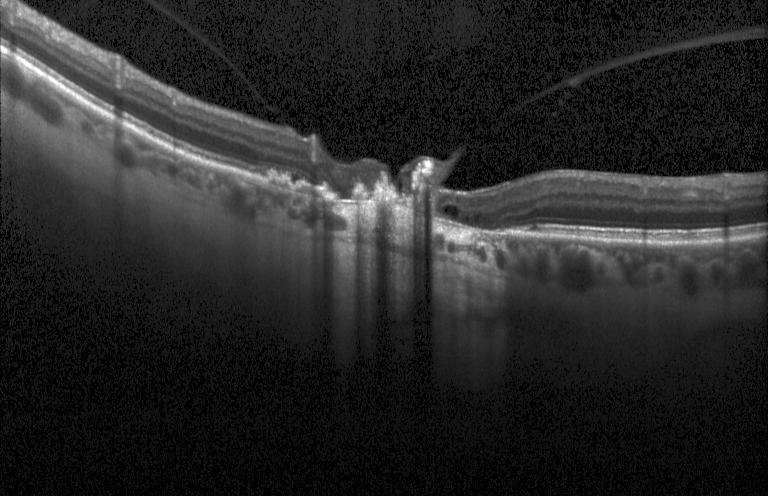
Retinal OCT cross-section. SD-OCT. Heidelberg Spectralis. Horizontal scan through the fovea.
Macular OCT: choroidal neovascularization.